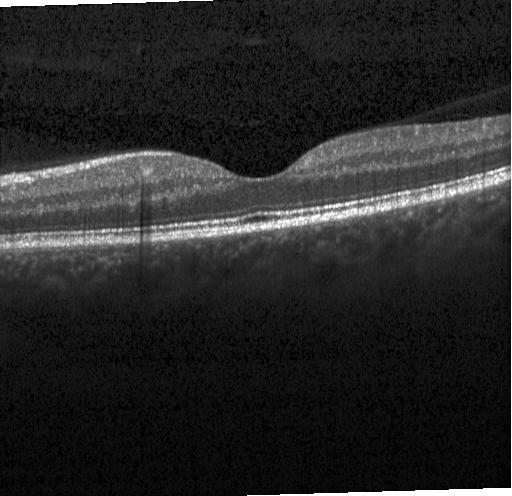

Retinal OCT B-scan. Dx: no choroidal neovascularization, no diabetic macular edema, and no drusen.